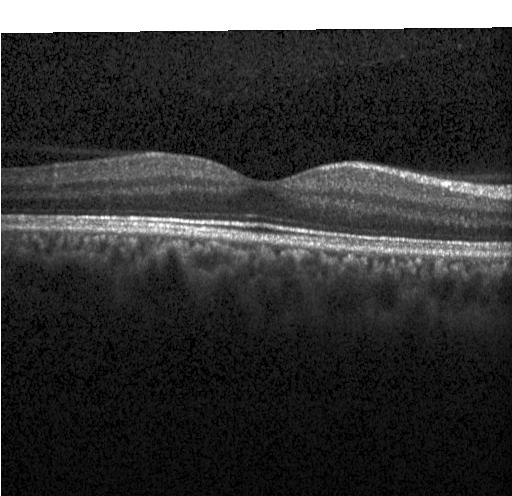

Centered on the fovea · SD-OCT · retinal OCT B-scan — Macular OCT: no choroidal neovascularization, diabetic macular edema, or drusen.